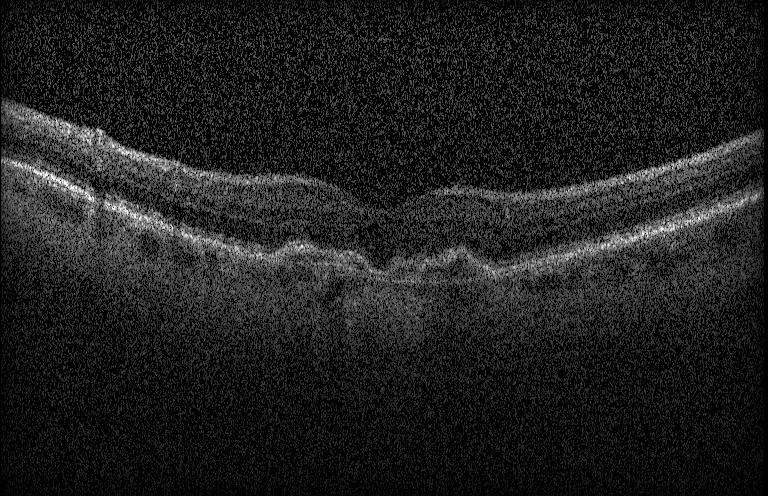 A choroidal neovascular membrane.